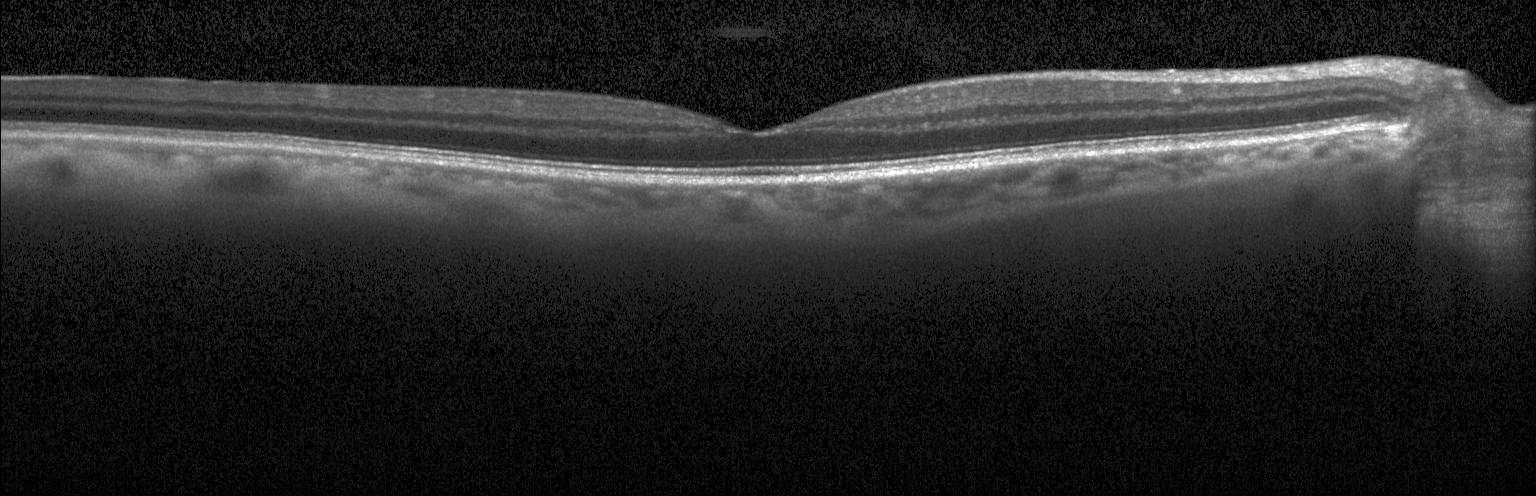

Horizontal scan through the fovea · spectral-domain optical coherence tomography · OCT B-scan · acquired on a Heidelberg Spectralis.
No choroidal neovascularization, diabetic macular edema, or drusen.